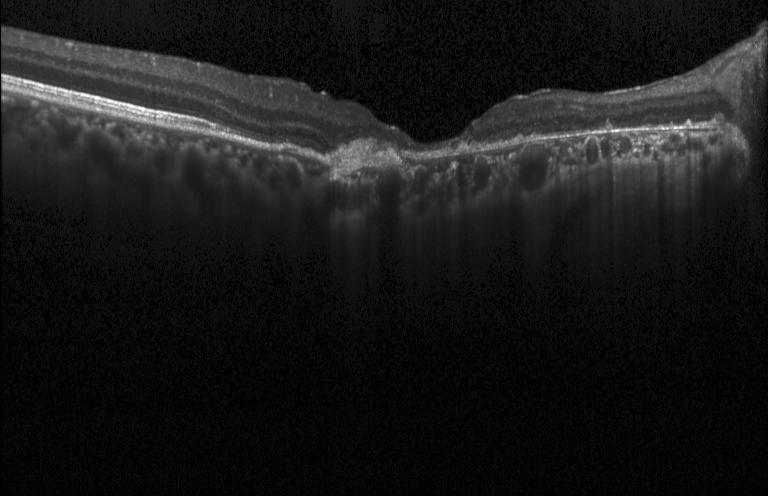

Diagnosis: choroidal neovascularization (CNV).